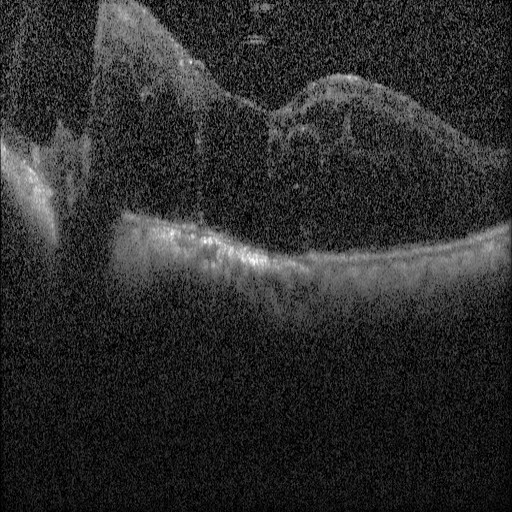

Diagnosis: DME.